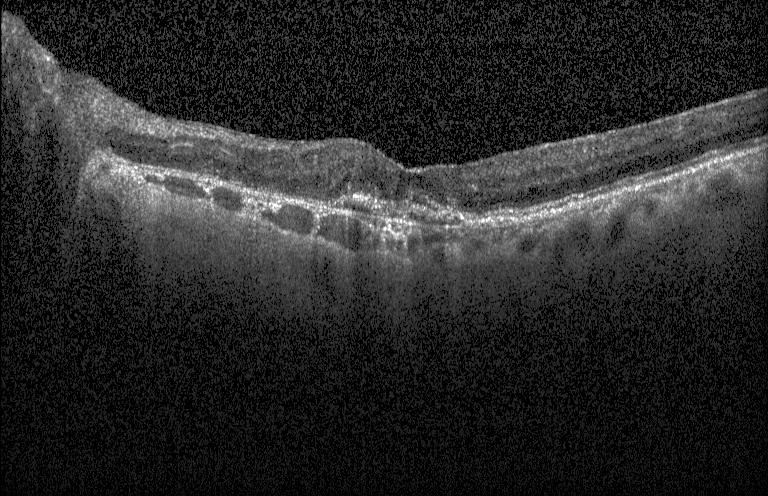

The scan shows a choroidal neovascular membrane.